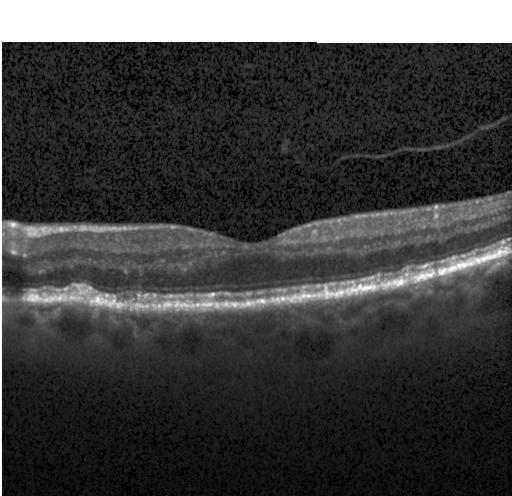 SD-OCT, retinal OCT cross-section, acquired on a Heidelberg Spectralis. Sub-RPE drusenoid deposits.